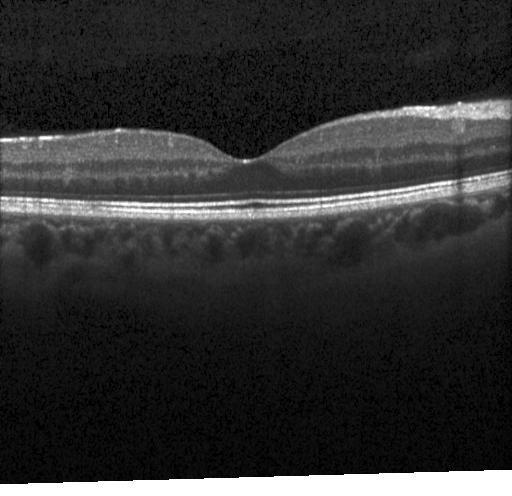 Assessment: no evidence of CNV, DME, or drusen.